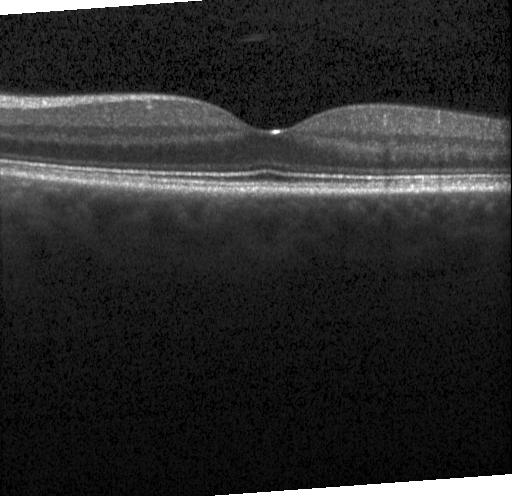 Retinal OCT cross-section — The scan shows no choroidal neovascularization, no diabetic macular edema, and no drusen.